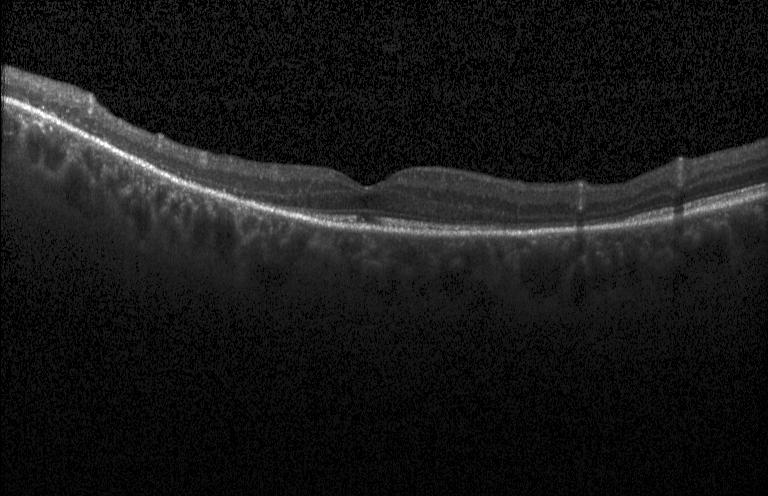 Impression: no evidence of choroidal neovascularization, diabetic macular edema, or drusen.